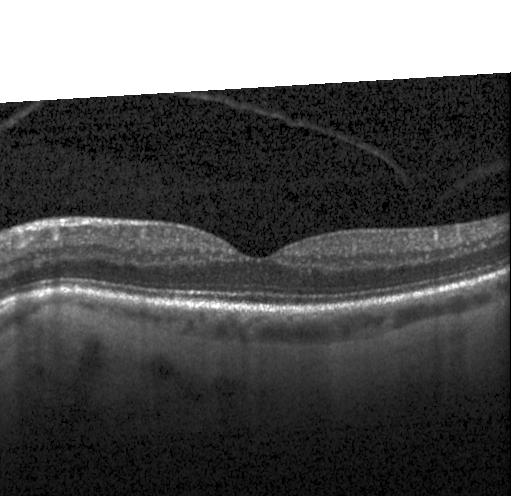 Diagnosis: no CNV, DME, or drusen.